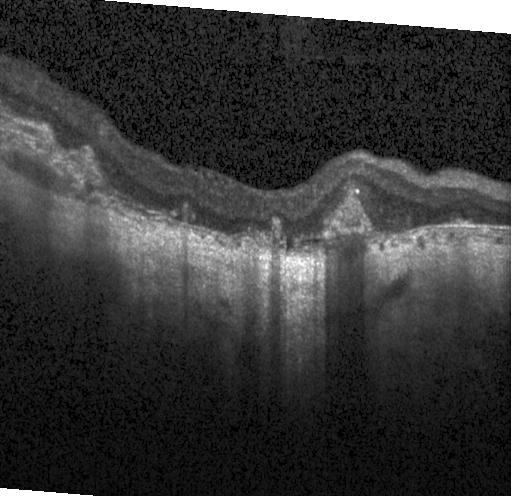 Impression: choroidal neovascularization (CNV).